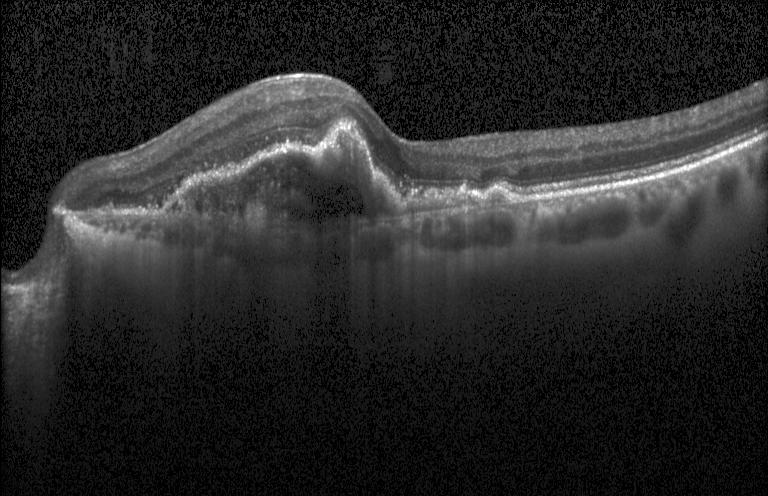
Through the macula. Spectral-domain OCT. Retinal OCT cross-section.
Choroidal neovascularization.